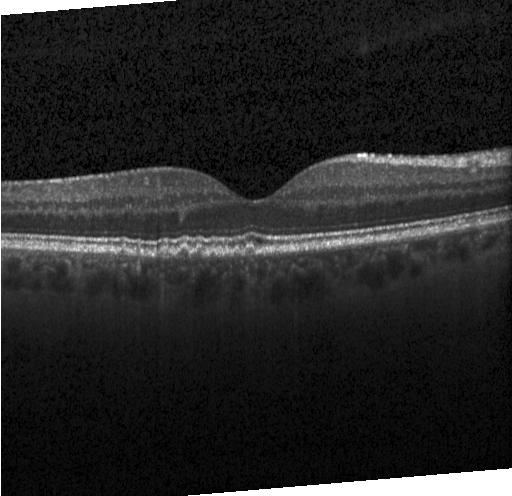 SD-OCT · optical coherence tomography scan · Heidelberg Spectralis OCT system · fovea-centered. Macular OCT: multiple drusen.